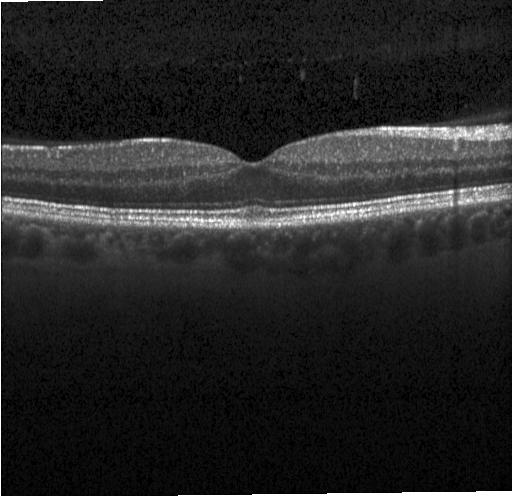
Finding: no evidence of choroidal neovascularization, diabetic macular edema, or drusen.